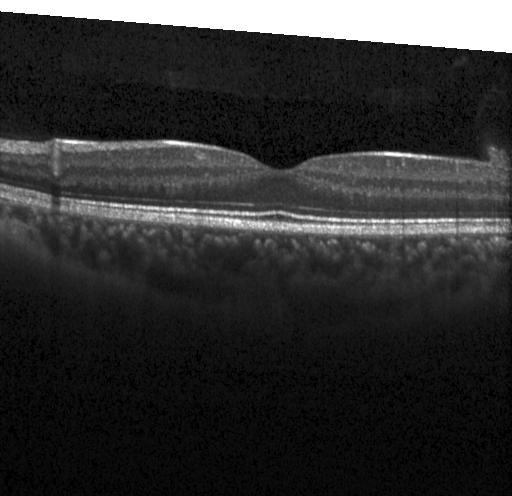
Dx: no evidence of choroidal neovascularization, diabetic macular edema, or drusen.